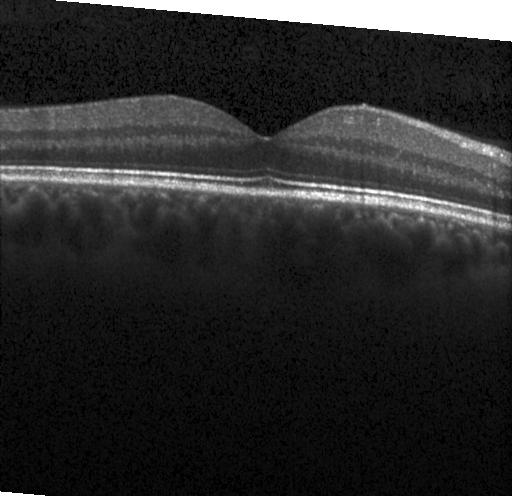
Optical coherence tomography B-scan, fovea-centered, Heidelberg Spectralis — Impression: no choroidal neovascularization, no diabetic macular edema, and no drusen.